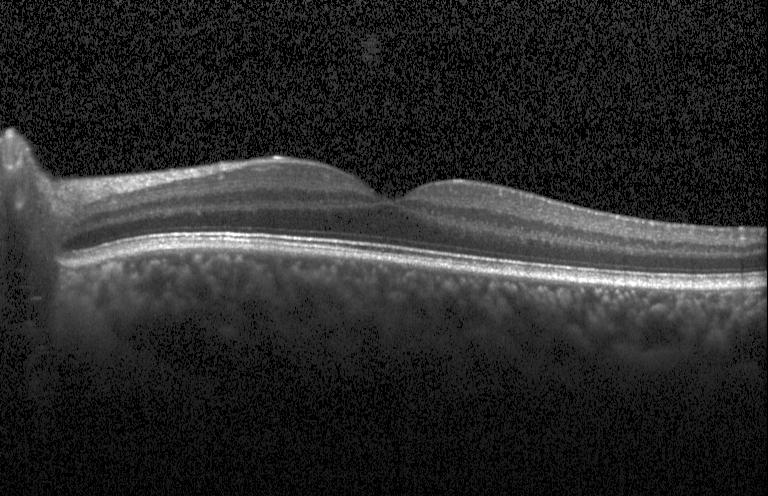

Diagnosis: no choroidal neovascularization, diabetic macular edema, or drusen.